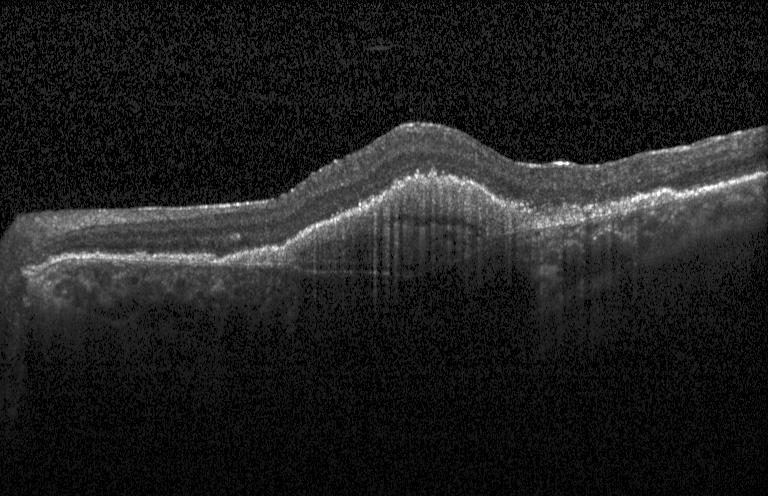
Finding: a choroidal neovascular membrane.